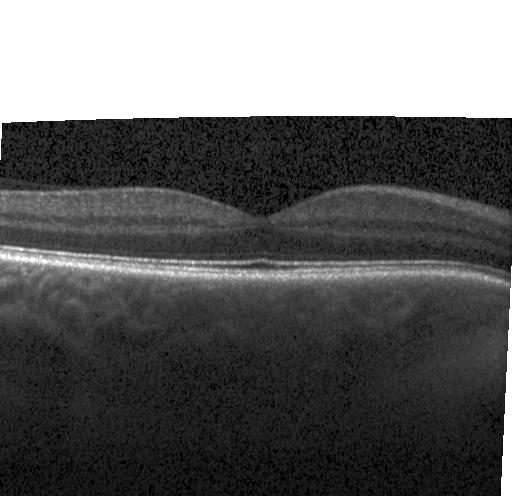 Neither choroidal neovascularization, diabetic macular edema, nor drusen.